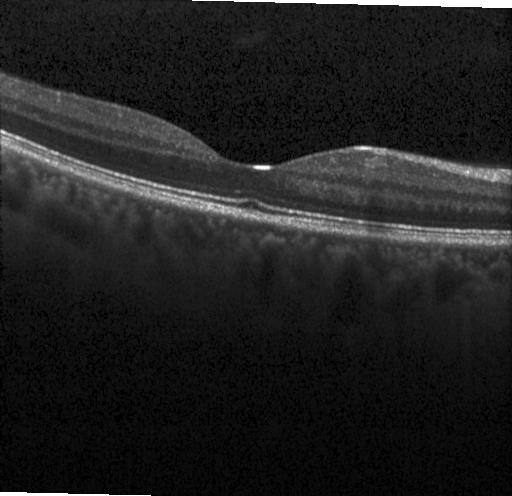
OCT B-scan showing no evidence of choroidal neovascularization, diabetic macular edema, or drusen.